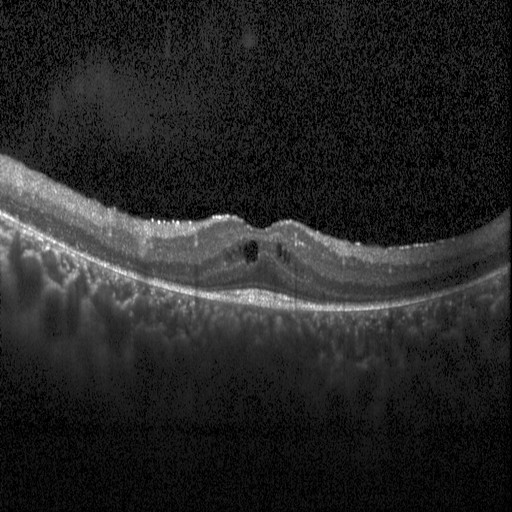

Spectral-domain optical coherence tomography · centered on the fovea · acquired on a Heidelberg Spectralis · OCT B-scan.
Diabetic macular edema (DME).